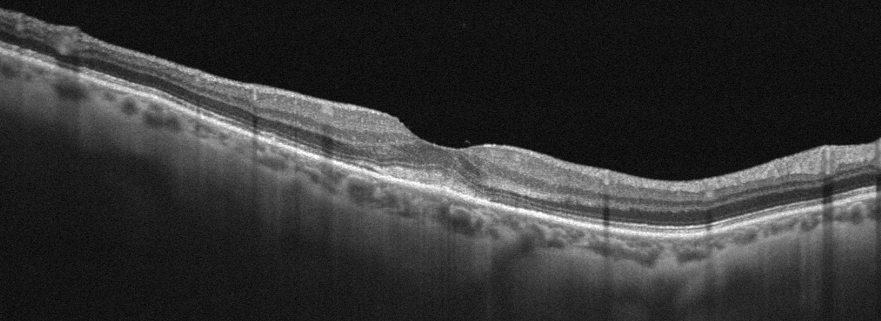

Macular OCT demonstrating age-related macular degeneration.